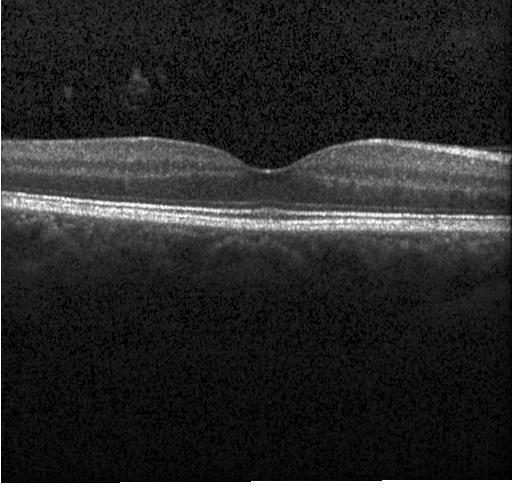 Optical coherence tomography B-scan, centered on the fovea, Heidelberg Spectralis OCT system.
Impression: no evidence of choroidal neovascularization, diabetic macular edema, or drusen.